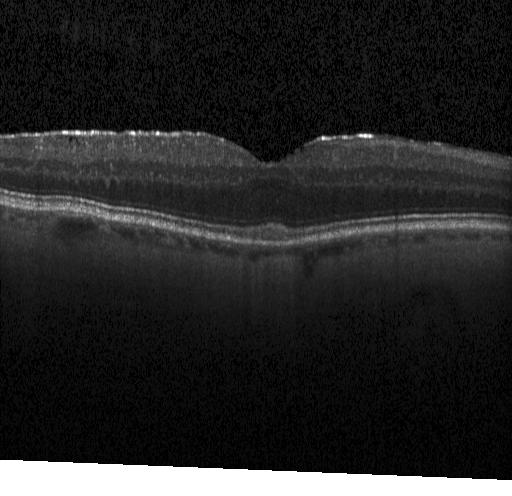
Retinal OCT B-scan. Macular OCT: drusen.